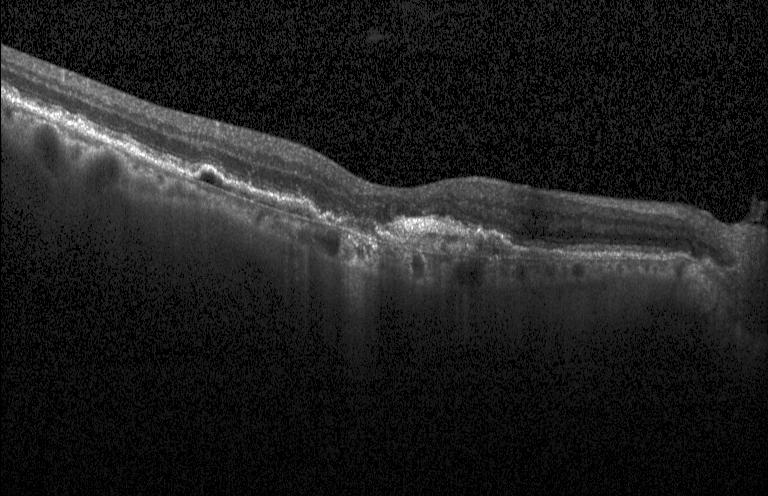 Macular OCT: a choroidal neovascular membrane.